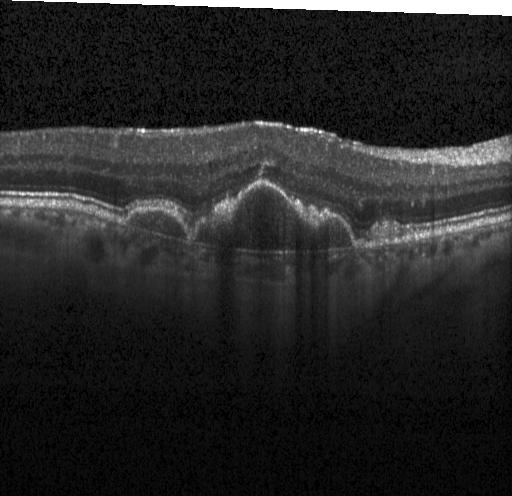
OCT finding: a choroidal neovascular membrane.